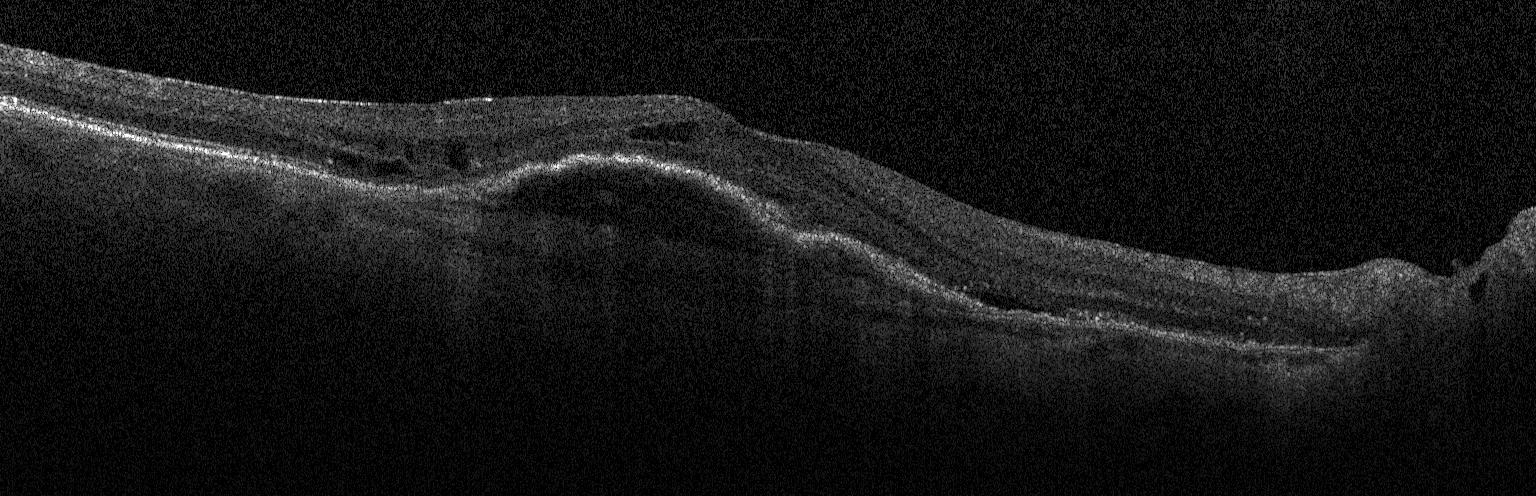

Retinal OCT cross-section; Heidelberg Spectralis — Finding: a choroidal neovascular membrane.